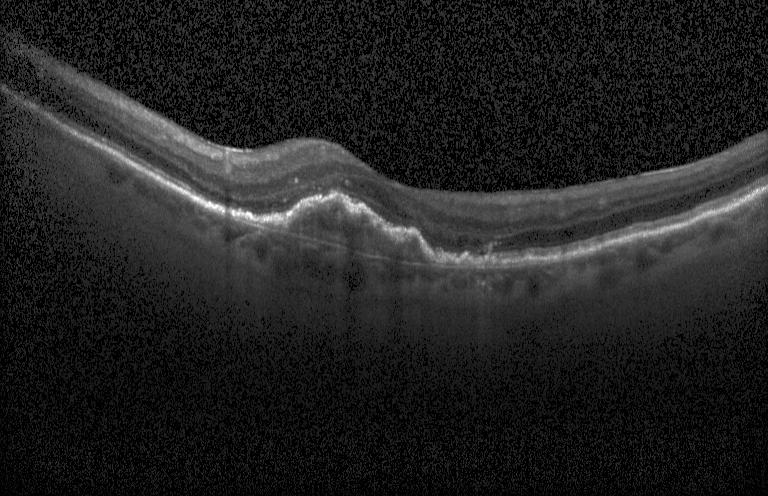 Impression: choroidal neovascularization.